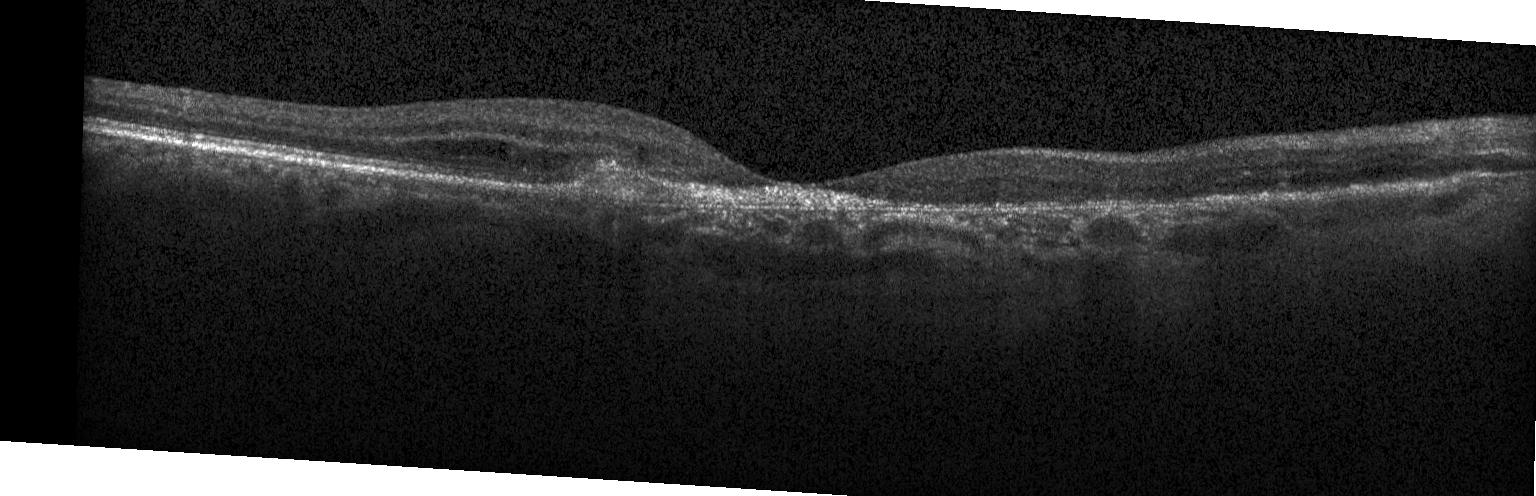
OCT line scan. This B-scan demonstrates CNV.